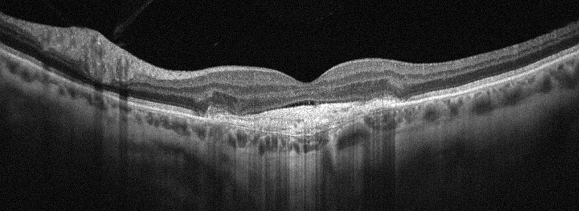
Left eye. OCT B-scan. Optovue Avanti RTVue XR. Macular scan. The scan shows age-related macular degeneration.